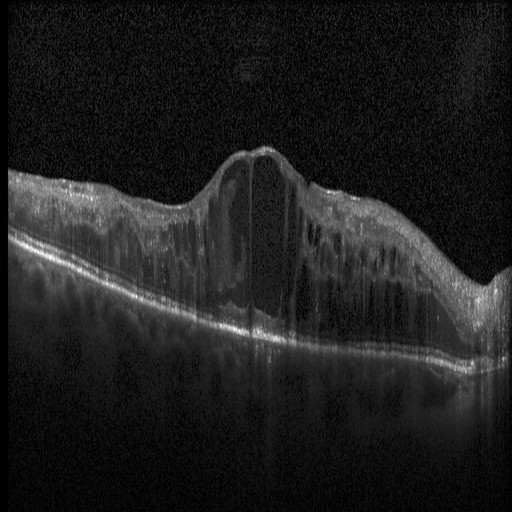

OCT line scan; Heidelberg Spectralis. Assessment: diabetic macular edema.